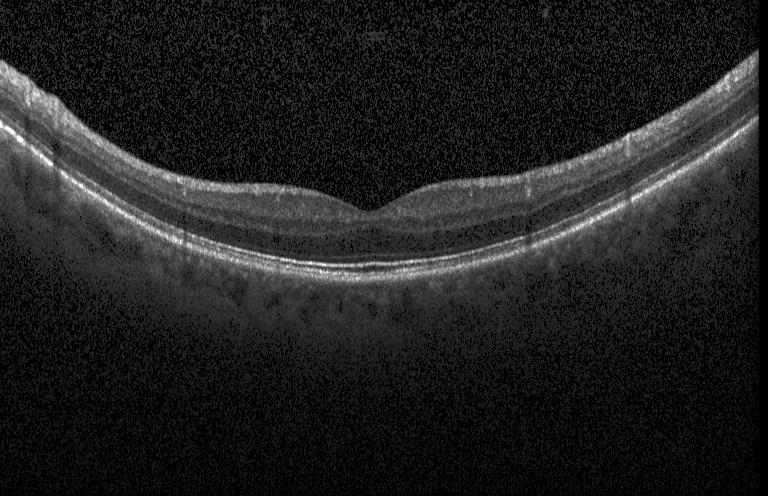 Acquired on a Heidelberg Spectralis, spectral-domain optical coherence tomography, fovea-centered, optical coherence tomography B-scan
Impression: no evidence of choroidal neovascularization, diabetic macular edema, or drusen.